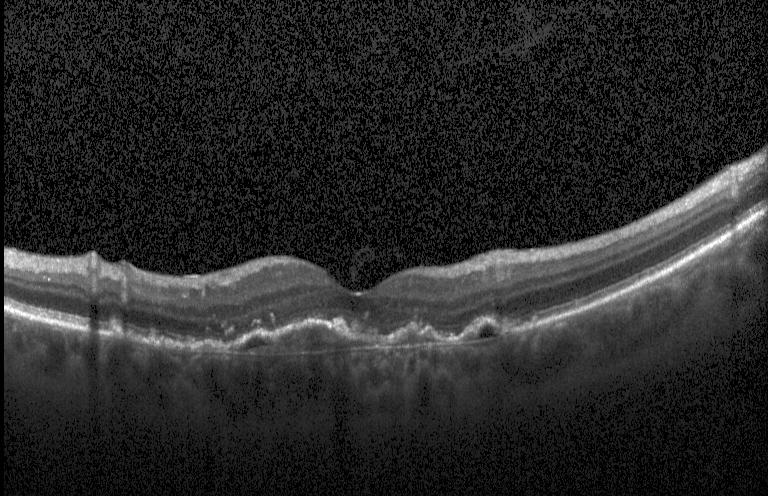

Spectral-domain optical coherence tomography; retinal OCT B-scan
Finding: choroidal neovascularization (CNV).